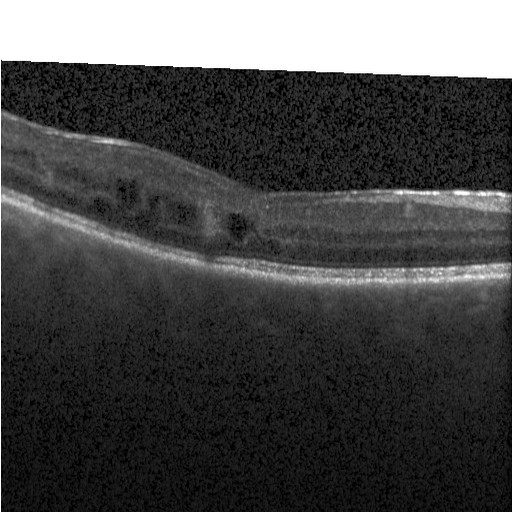 The scan shows diabetic macular edema (DME).